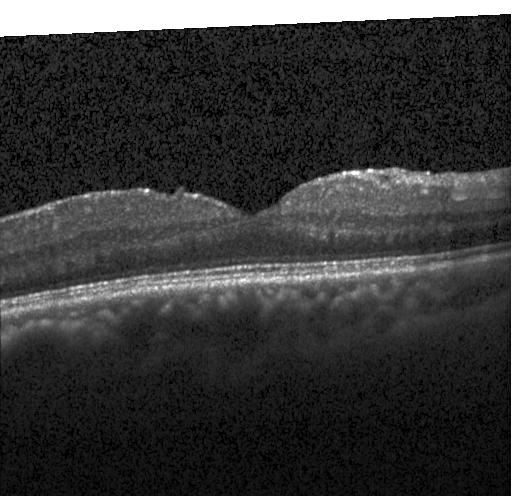

OCT line scan — Diagnosis: no choroidal neovascularization, no diabetic macular edema, and no drusen.